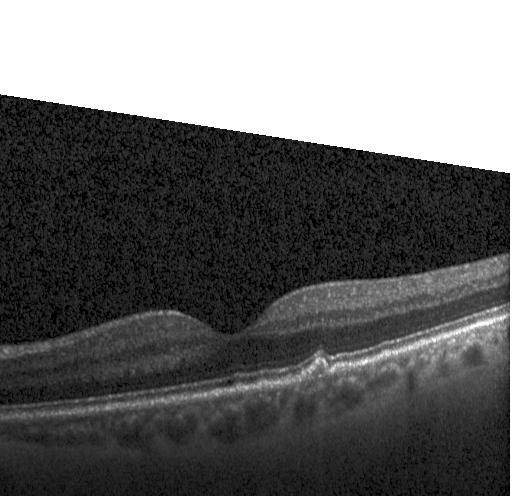 Retinal OCT cross-section
Multiple drusen.